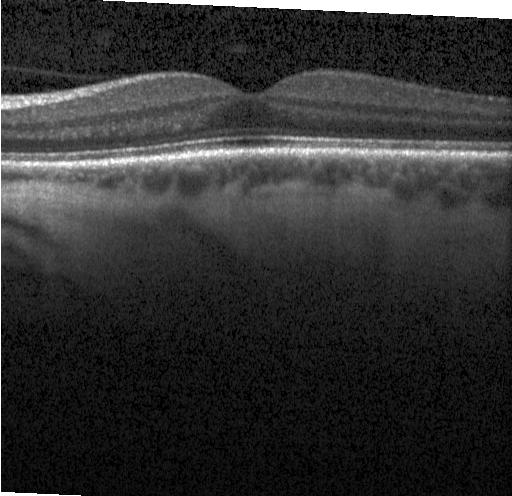 Finding: no CNV, DME, or drusen.